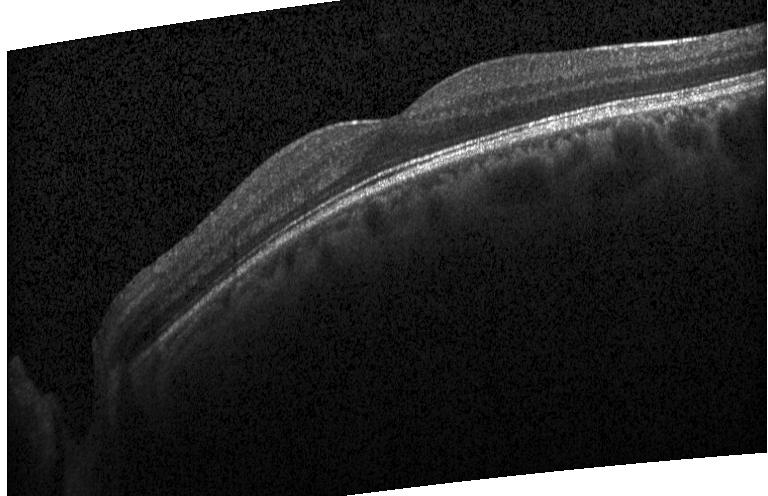

Optical coherence tomography scan — Finding: neither choroidal neovascularization, diabetic macular edema, nor drusen.